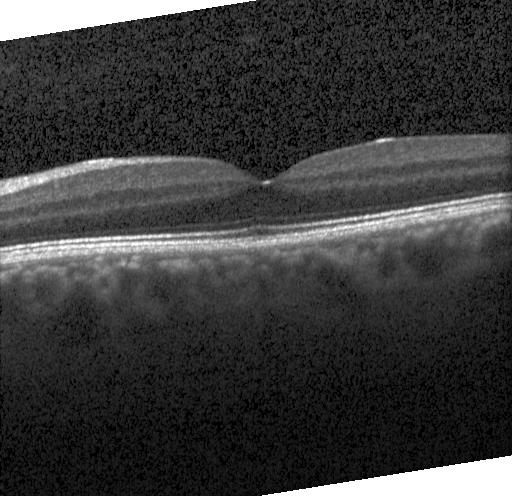

Optical coherence tomography B-scan; SD-OCT; Heidelberg Spectralis OCT system. Macular OCT: no choroidal neovascularization, no diabetic macular edema, and no drusen.